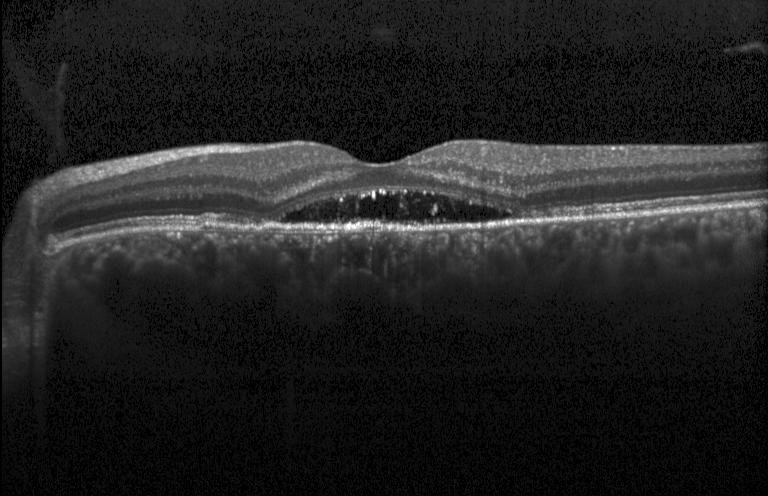 Horizontal scan through the fovea. Spectral-domain OCT. Acquired on a Heidelberg Spectralis. OCT line scan — Dx: CNV.